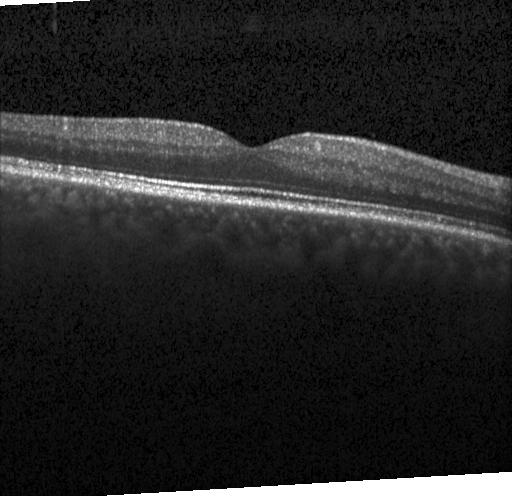 Retinal OCT cross-section. Diagnosis: no evidence of CNV, DME, or drusen.